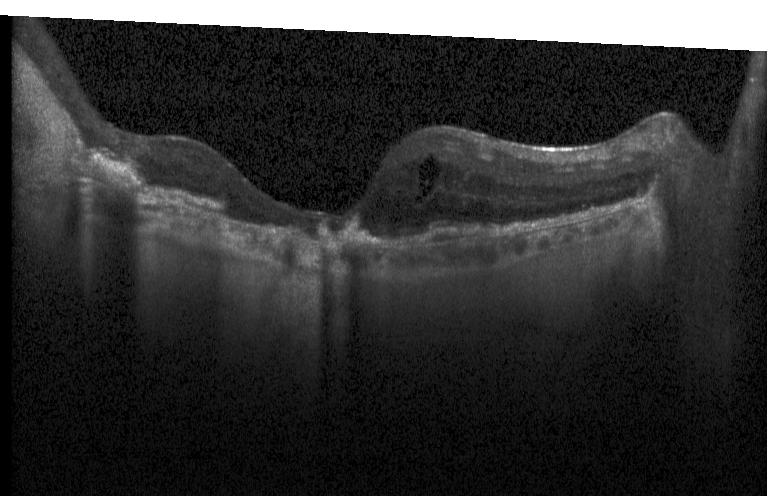 Dx: a choroidal neovascular membrane.